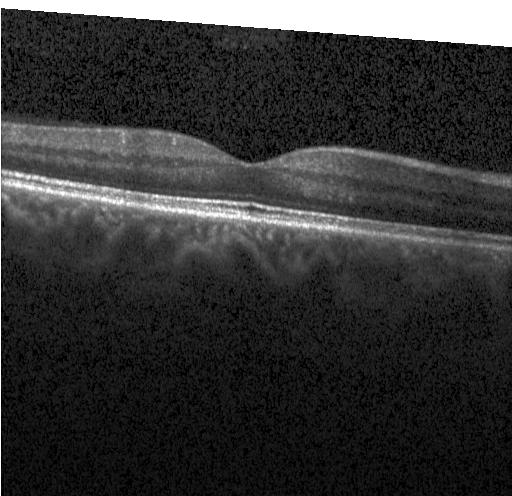
Retinal OCT cross-section — No CNV, DME, or drusen.